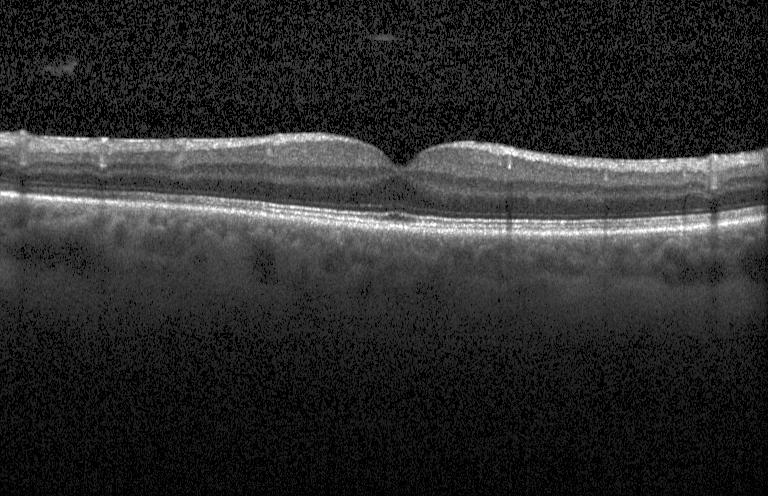

Heidelberg Spectralis, OCT B-scan. This B-scan demonstrates neither CNV, DME, nor drusen.